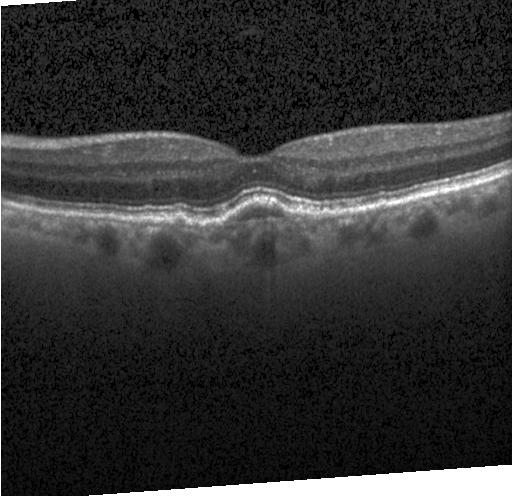

Heidelberg Spectralis OCT system; retinal OCT B-scan. Finding: a choroidal neovascular membrane.